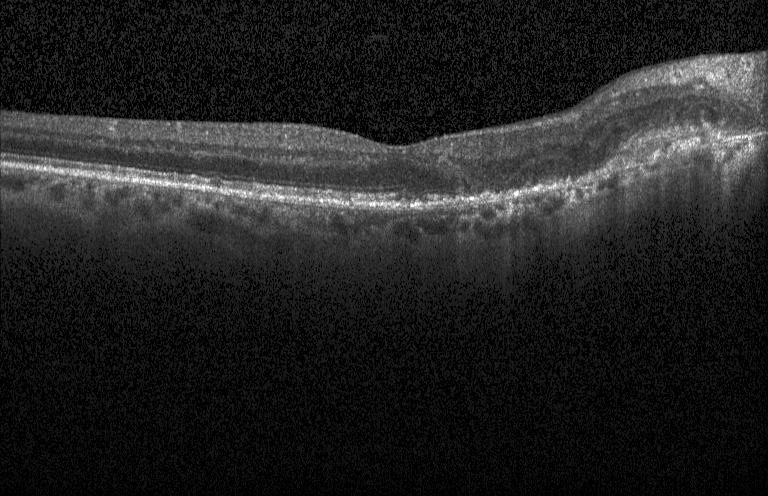
Macular OCT demonstrating CNV.